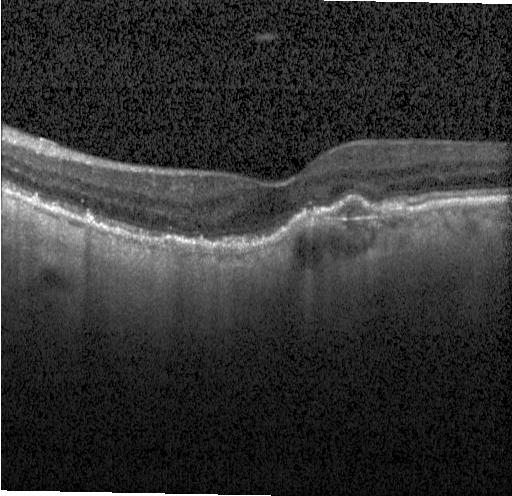

Spectral-domain OCT. Retinal OCT B-scan. Instrument: Heidelberg Spectralis
Finding: choroidal neovascularization (CNV).